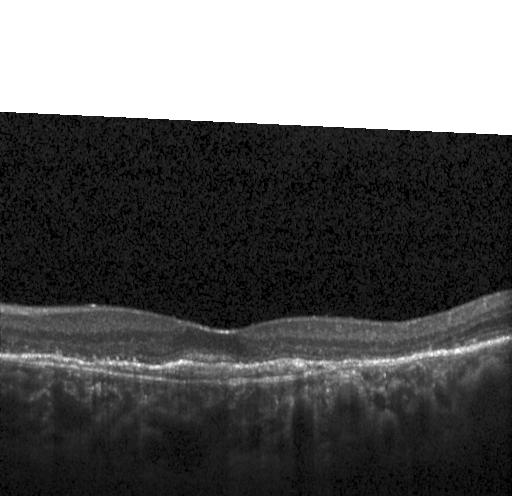
Spectral-domain optical coherence tomography, optical coherence tomography B-scan
Diagnosis: a choroidal neovascular membrane.